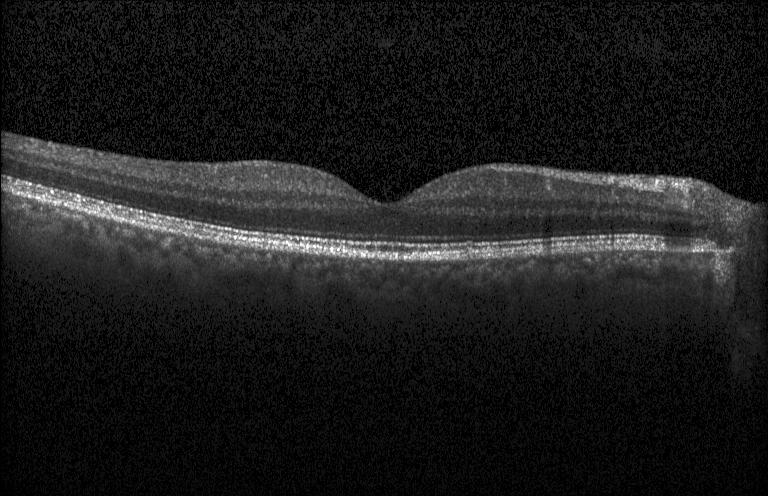
This B-scan demonstrates no choroidal neovascularization, diabetic macular edema, or drusen.